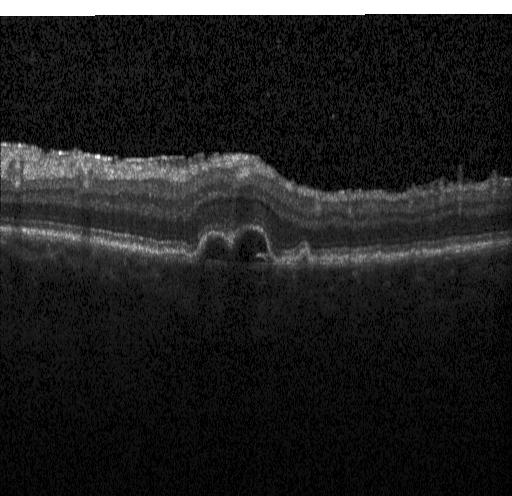
Retinal OCT B-scan.
Impression: a choroidal neovascular membrane.